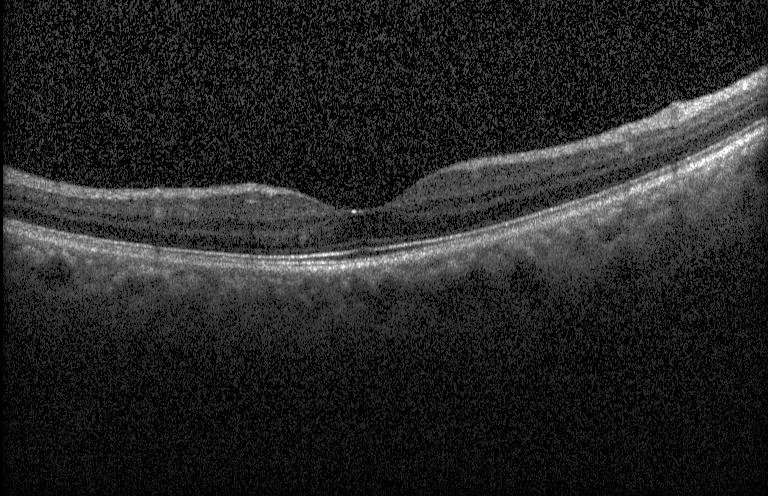
Macular OCT demonstrating no choroidal neovascularization, diabetic macular edema, or drusen.